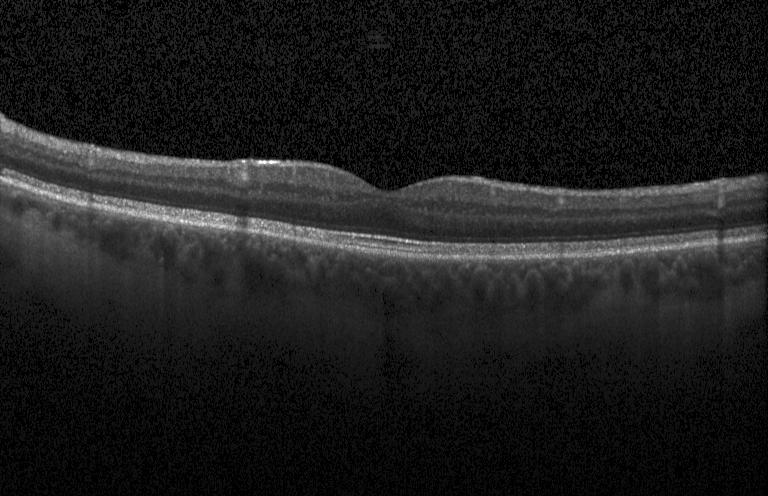

Spectral-domain optical coherence tomography, retinal OCT cross-section. No evidence of choroidal neovascularization, diabetic macular edema, or drusen.